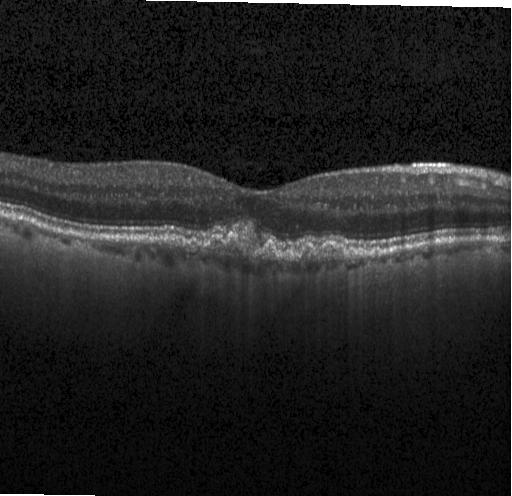

Retinal OCT cross-section; centered on the fovea — The scan shows sub-RPE drusenoid deposits.